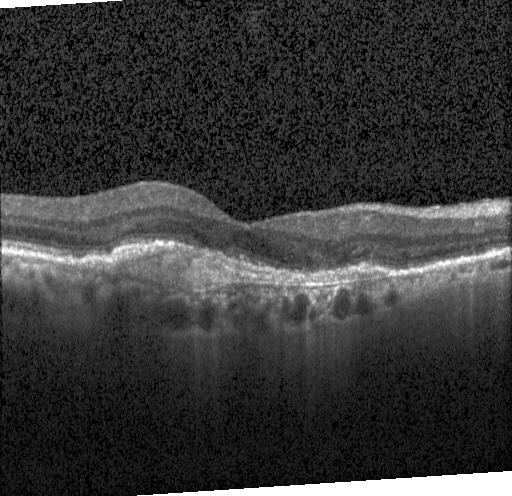
Optical coherence tomography B-scan. Horizontal scan through the fovea. Spectral-domain optical coherence tomography. Heidelberg Spectralis.
Finding: choroidal neovascularization (CNV).